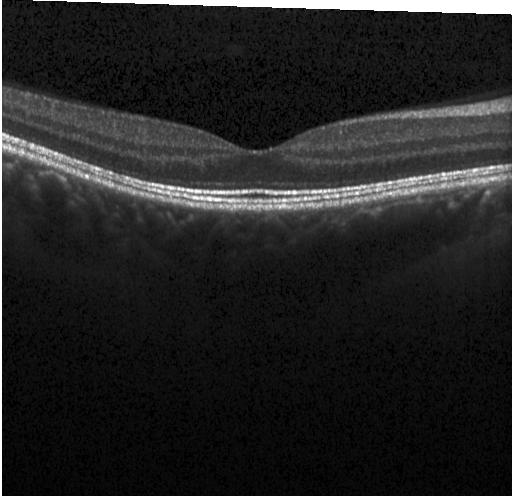

Macular OCT demonstrating no choroidal neovascularization, diabetic macular edema, or drusen.